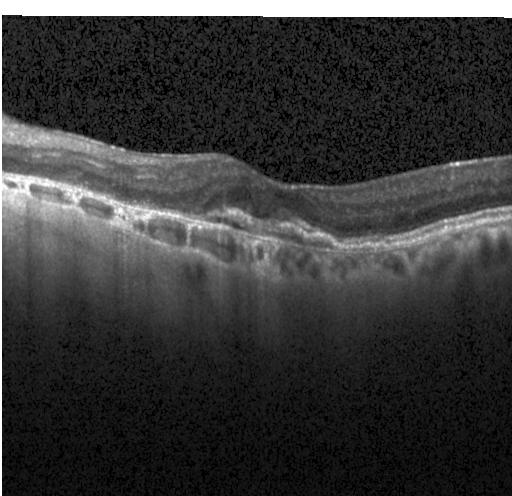

OCT B-scan — OCT finding: choroidal neovascularization.